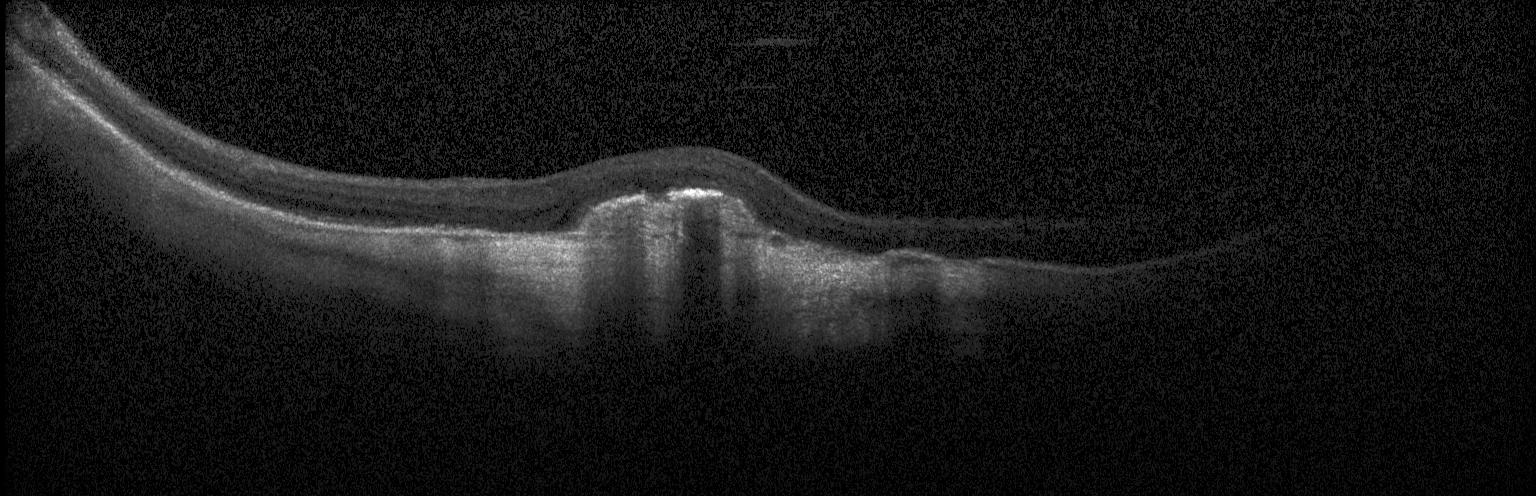

Macular OCT: a choroidal neovascular membrane.